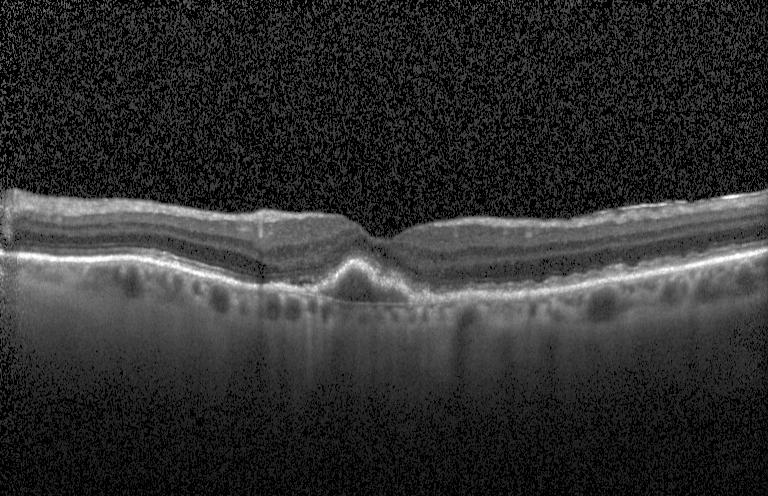 Centered on the fovea, retinal OCT B-scan — Diagnosis: choroidal neovascularization (CNV).